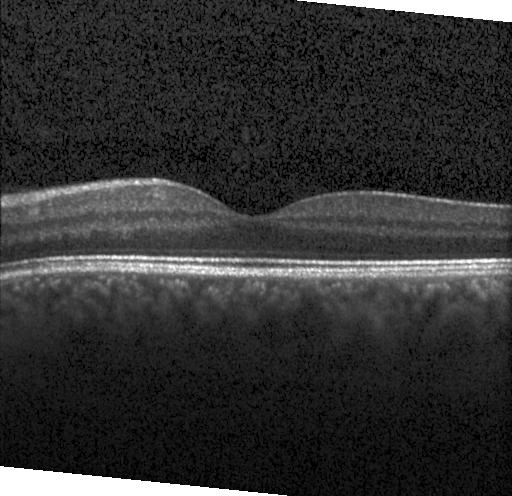
Diagnosis: neither choroidal neovascularization, diabetic macular edema, nor drusen.